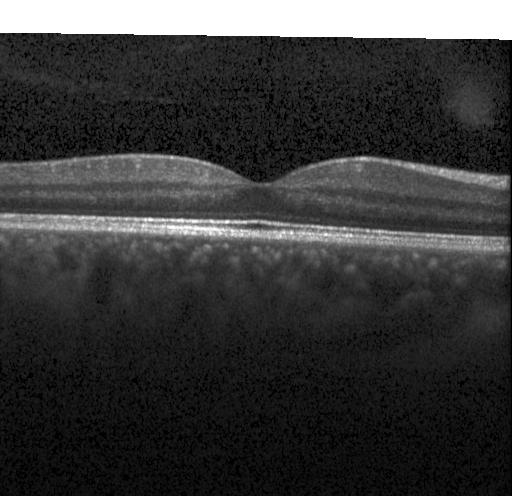
Impression: no evidence of choroidal neovascularization, diabetic macular edema, or drusen.